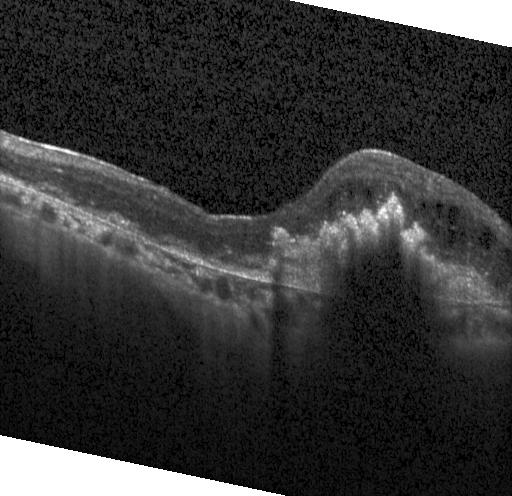
Instrument: Heidelberg Spectralis, retinal OCT cross-section, SD-OCT
CNV.